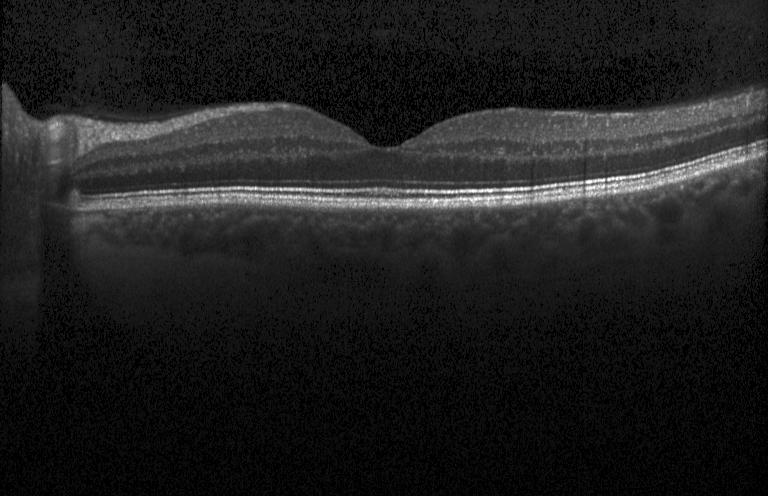 Retinal OCT cross-section.
Diagnosis: no evidence of choroidal neovascularization, diabetic macular edema, or drusen.